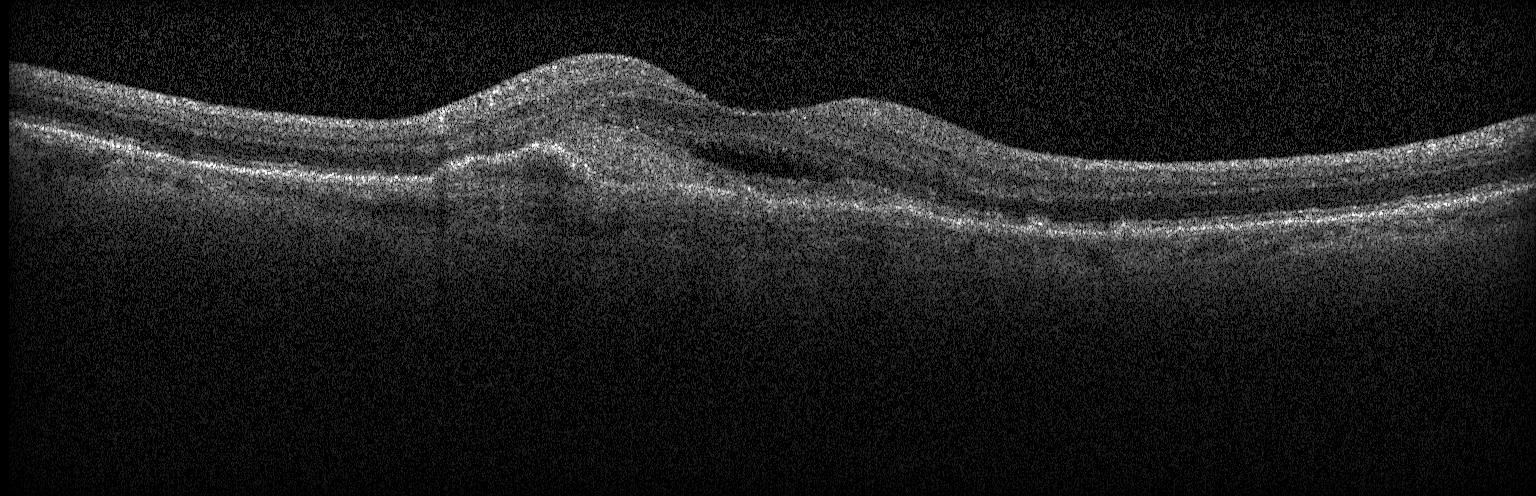

Spectral-domain OCT. OCT line scan. Macular scan. Acquired on a Heidelberg Spectralis. Finding: a choroidal neovascular membrane.